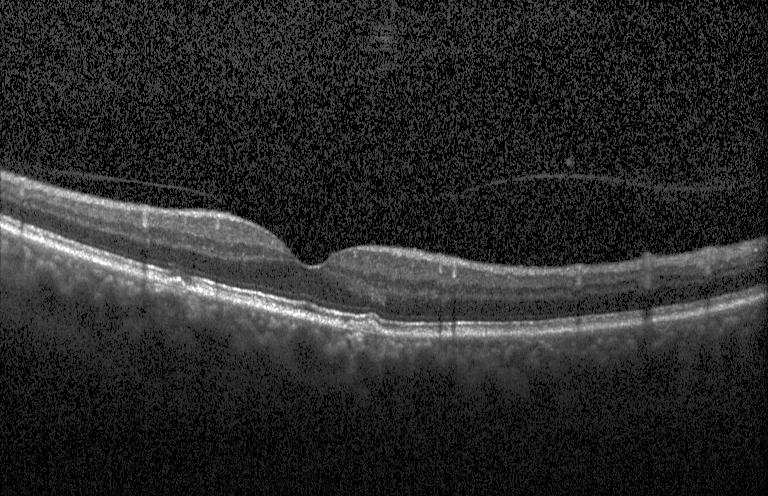 OCT B-scan, spectral-domain OCT, Heidelberg Spectralis — Diagnosis: multiple drusen.